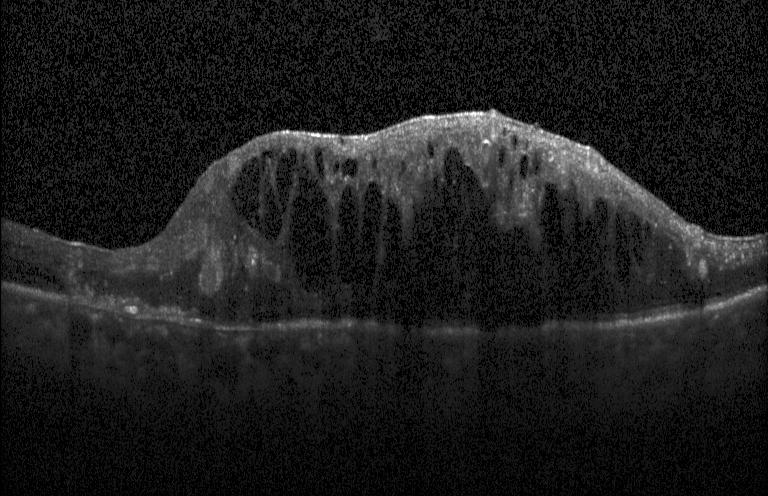 Through the macula; OCT line scan; SD-OCT; Heidelberg Spectralis. Diagnosis: diabetic macular edema.